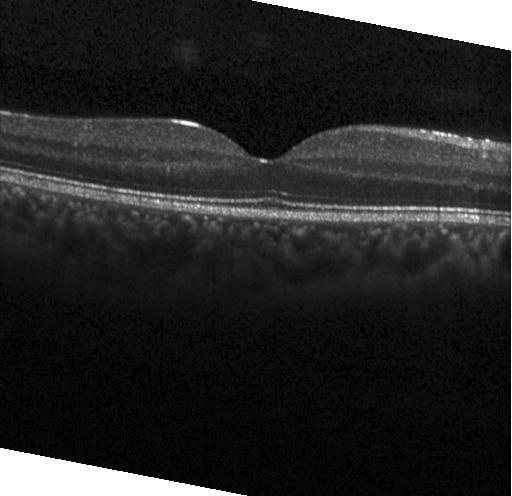 Macular OCT demonstrating neither choroidal neovascularization, diabetic macular edema, nor drusen.